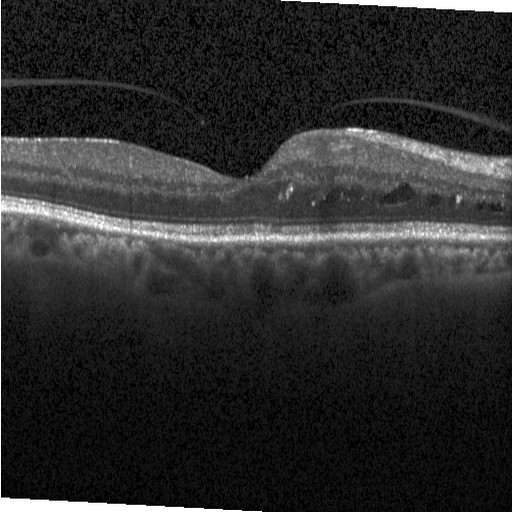

OCT scan showing diabetic macular edema.